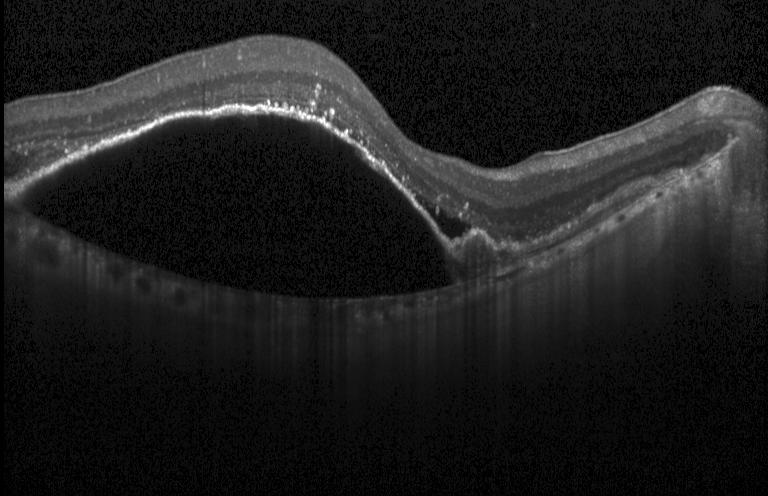 Spectral-domain OCT B-scan: CNV.